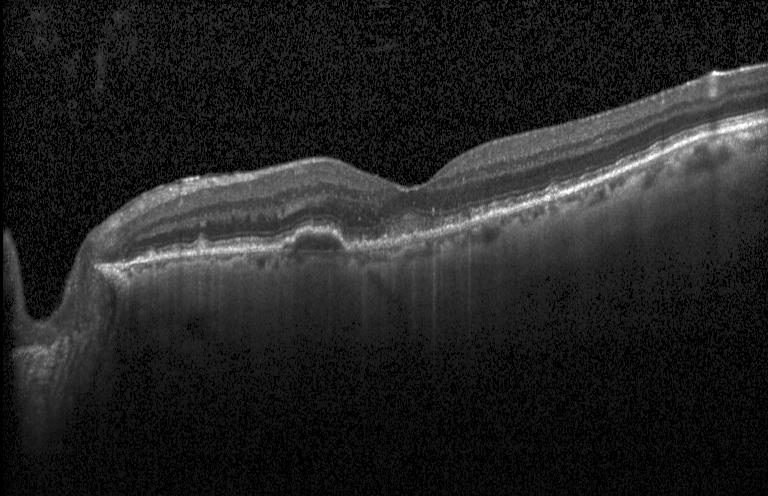 Spectral-domain OCT, retinal OCT cross-section
Finding: choroidal neovascularization.